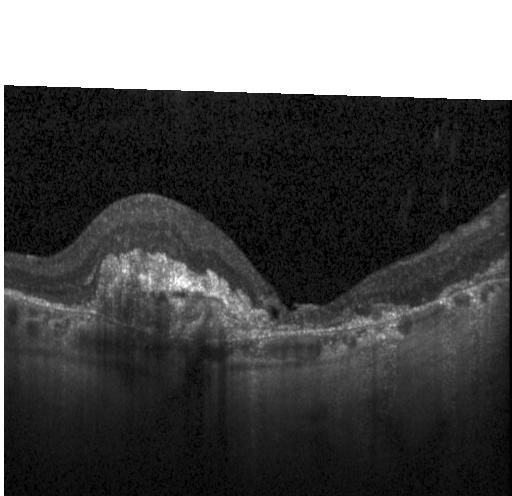 OCT line scan — Diagnosis: CNV.